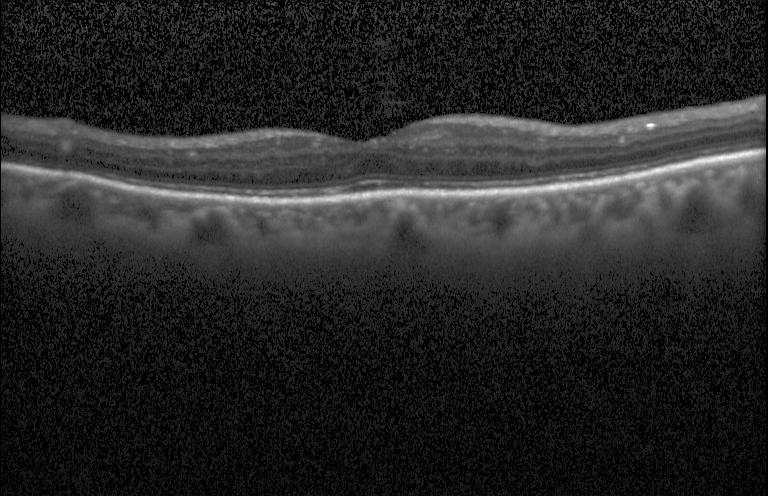
Heidelberg Spectralis. Retinal OCT B-scan — Finding: no choroidal neovascularization, no diabetic macular edema, and no drusen.